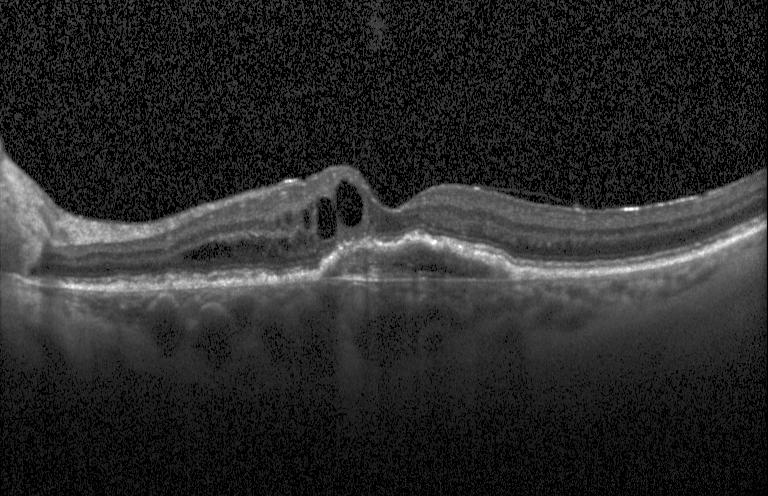

Diagnosis: choroidal neovascularization.